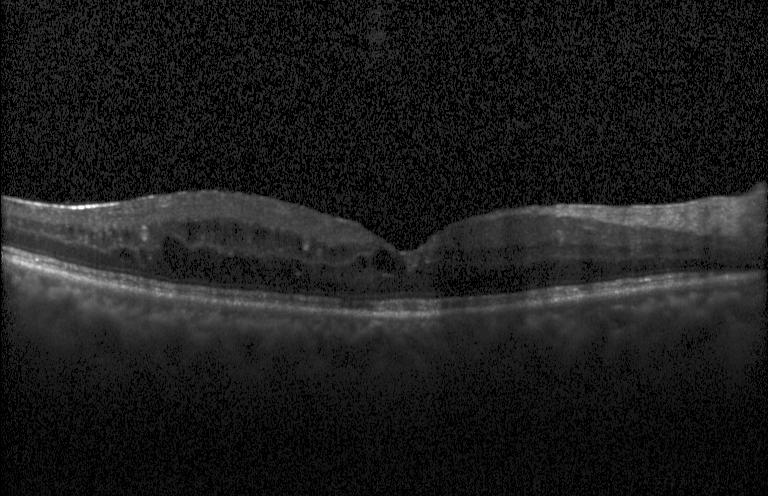

OCT finding: diabetic macular edema.